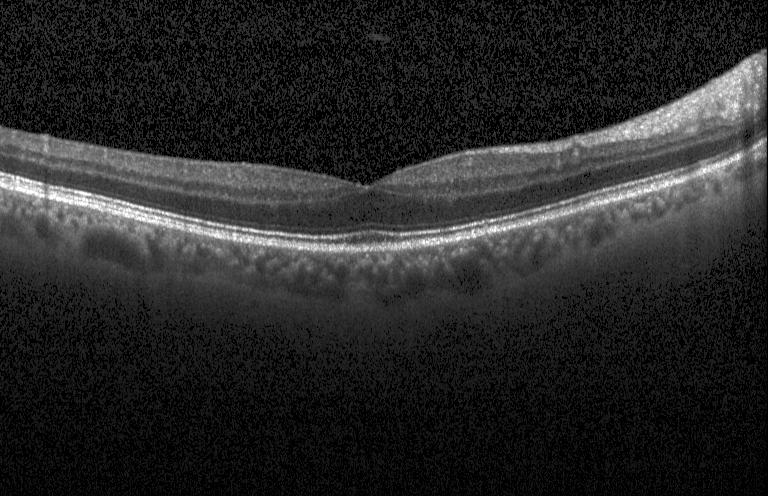
SD-OCT · optical coherence tomography B-scan · Heidelberg Spectralis · macular scan — Macular OCT: no choroidal neovascularization, diabetic macular edema, or drusen.